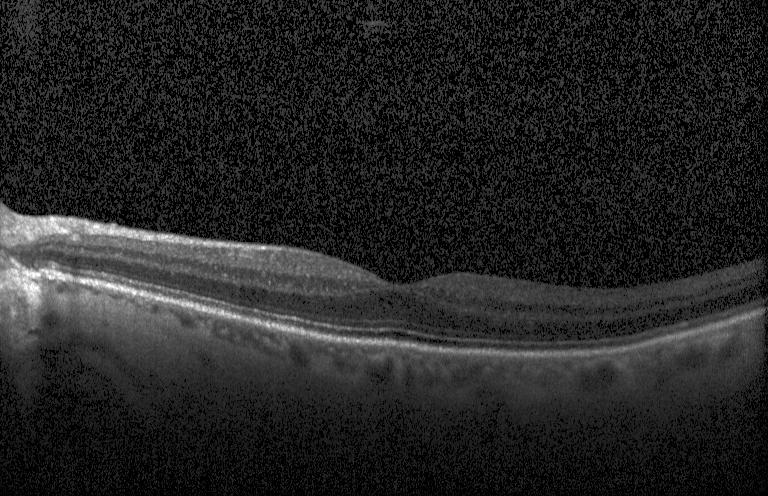

Acquired on a Heidelberg Spectralis · spectral-domain OCT · OCT line scan · through the macula. Macular OCT: no choroidal neovascularization, diabetic macular edema, or drusen.